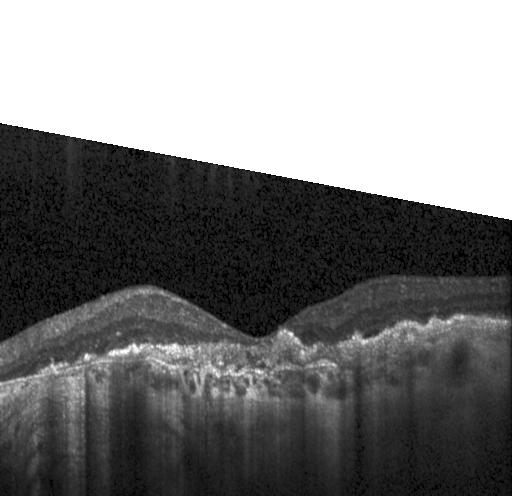 The scan shows CNV.